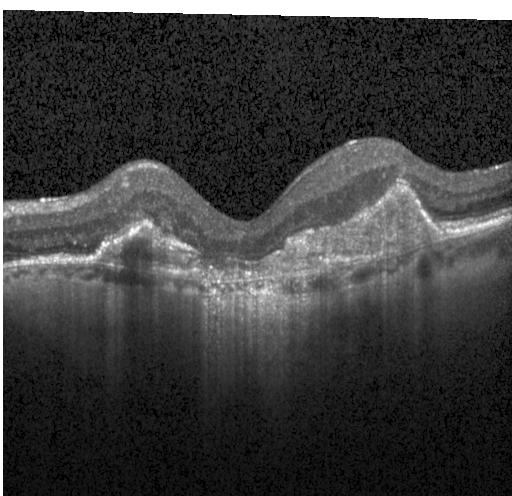

OCT scan showing CNV.